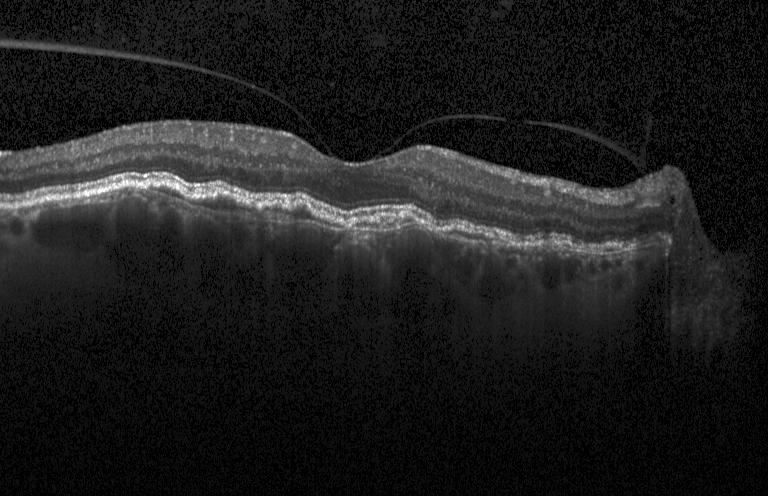

Optical coherence tomography scan. SD-OCT — Diagnosis: a choroidal neovascular membrane.